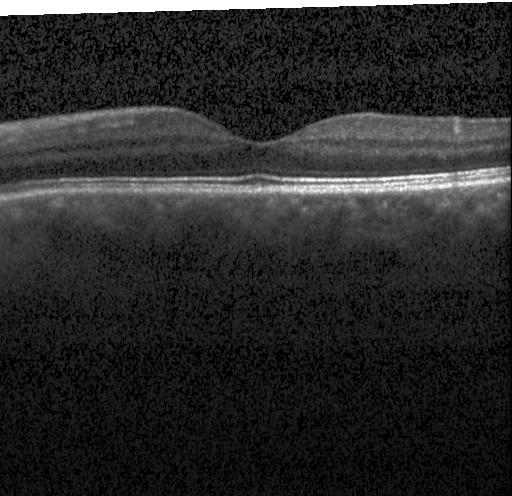
Impression: no CNV, no DME, and no drusen.